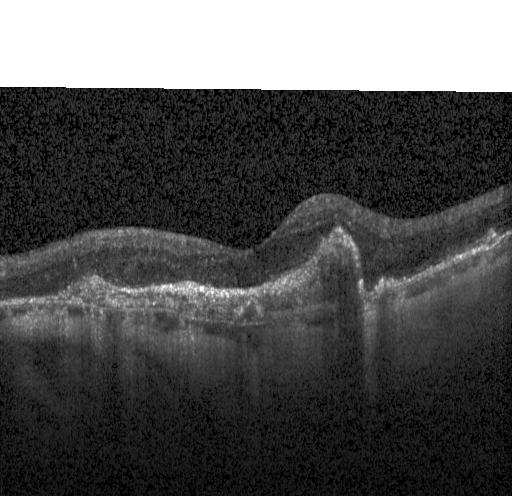
SD-OCT; horizontal scan through the fovea; optical coherence tomography scan — Dx: choroidal neovascularization (CNV).